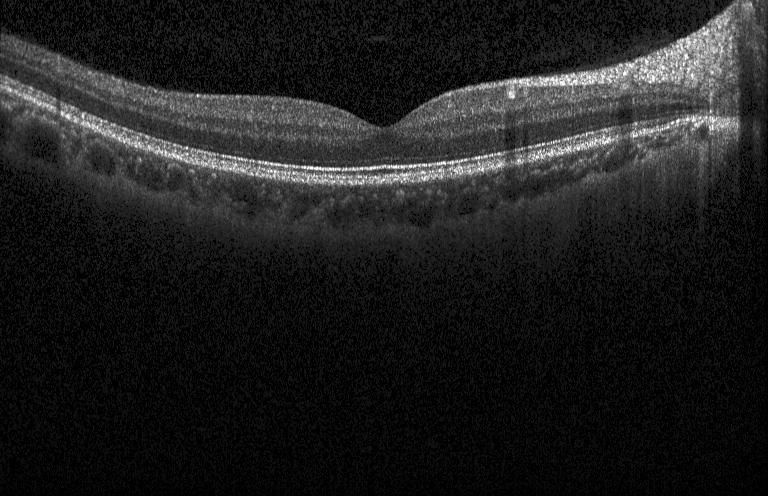

Finding: neither choroidal neovascularization, diabetic macular edema, nor drusen.